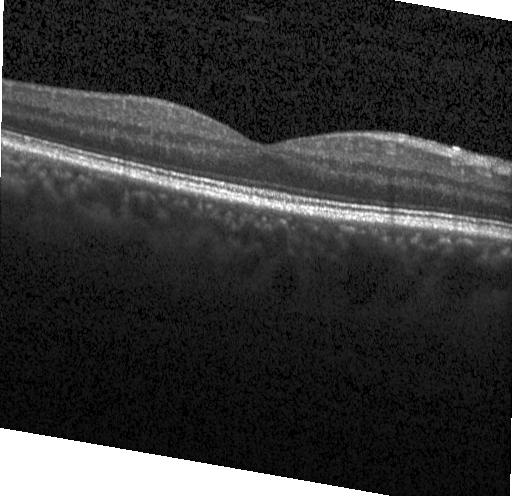
Impression: no choroidal neovascularization, no diabetic macular edema, and no drusen.